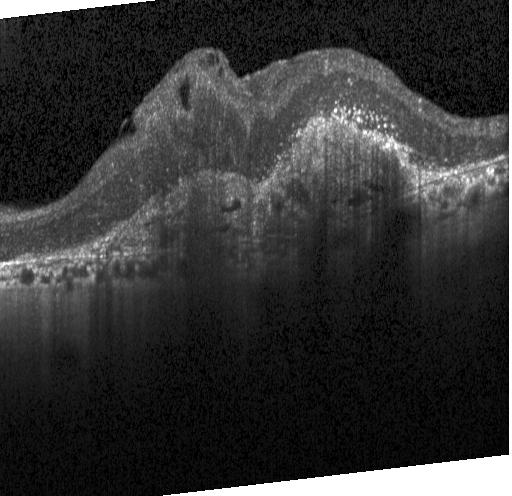

The scan shows CNV.